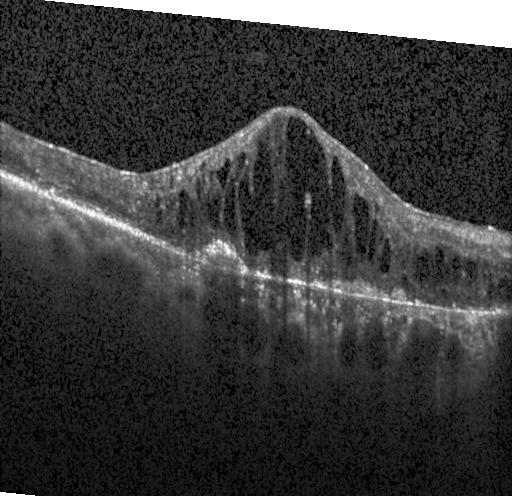 Macular scan. Optical coherence tomography B-scan — Finding: CNV.